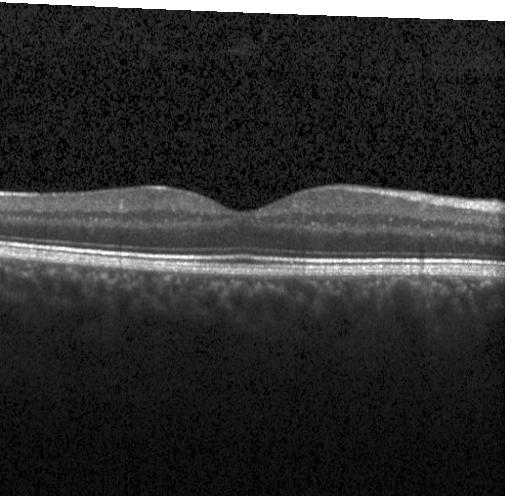 Macular OCT demonstrating no CNV, DME, or drusen.